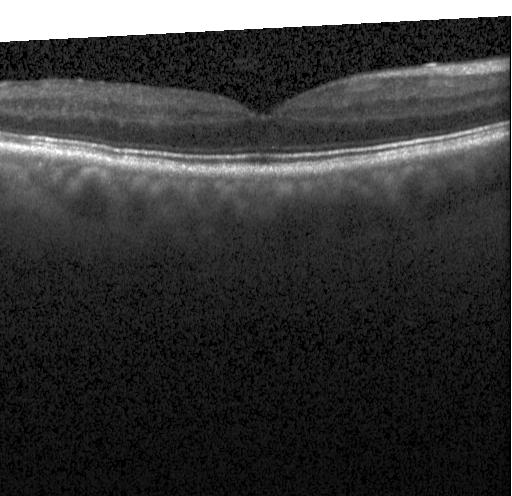

Optical coherence tomography B-scan
This B-scan demonstrates no CNV, no DME, and no drusen.